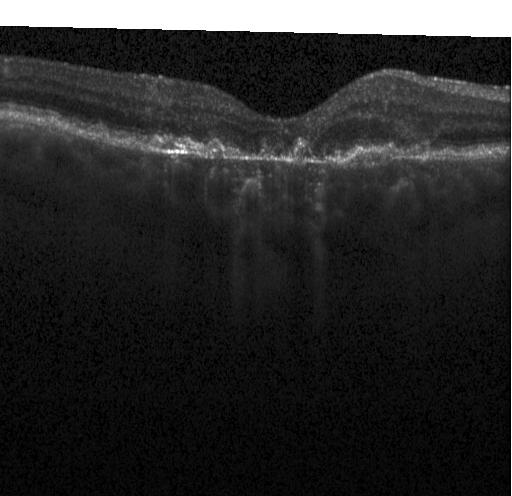

Spectral-domain OCT B-scan: choroidal neovascularization.